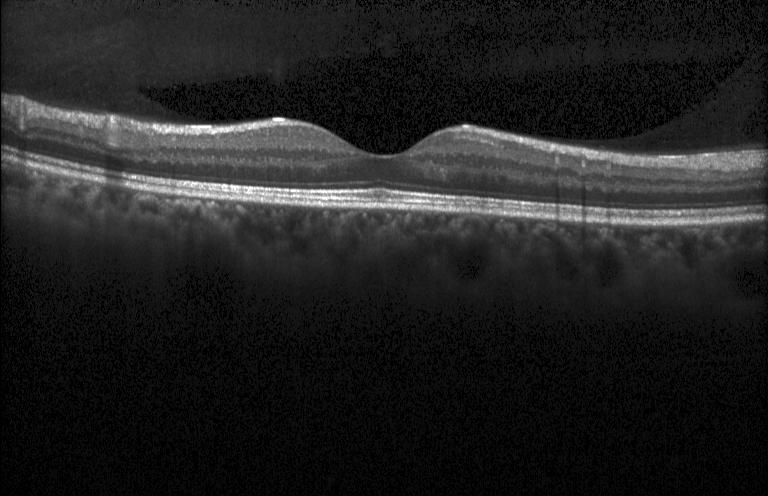

Optical coherence tomography B-scan.
No choroidal neovascularization, no diabetic macular edema, and no drusen.